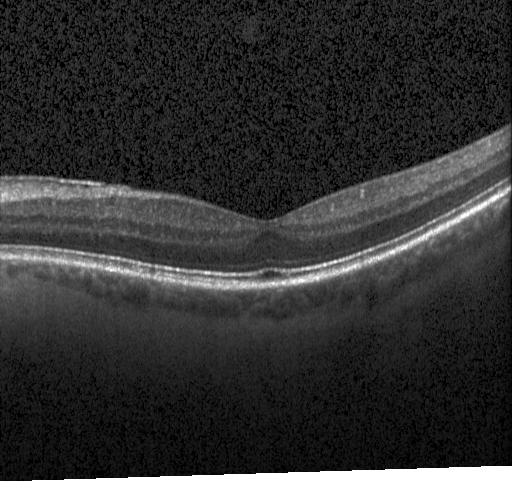

This B-scan demonstrates no CNV, DME, or drusen.